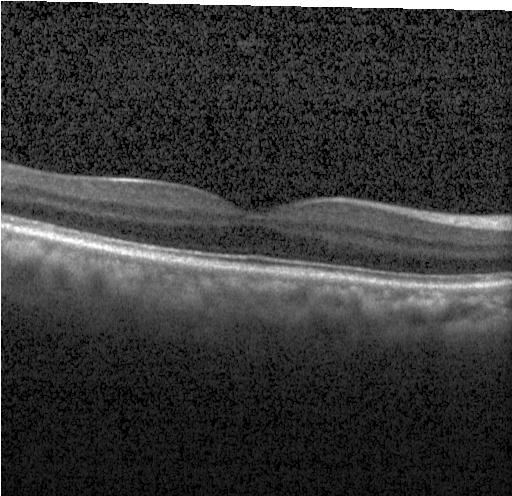
Diagnosis: no choroidal neovascularization, no diabetic macular edema, and no drusen.